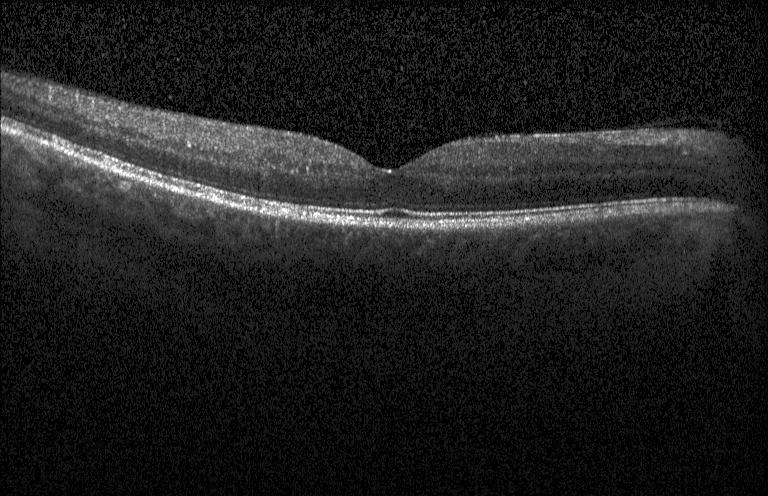
Optical coherence tomography B-scan · acquired on a Heidelberg Spectralis.
This B-scan demonstrates no CNV, DME, or drusen.